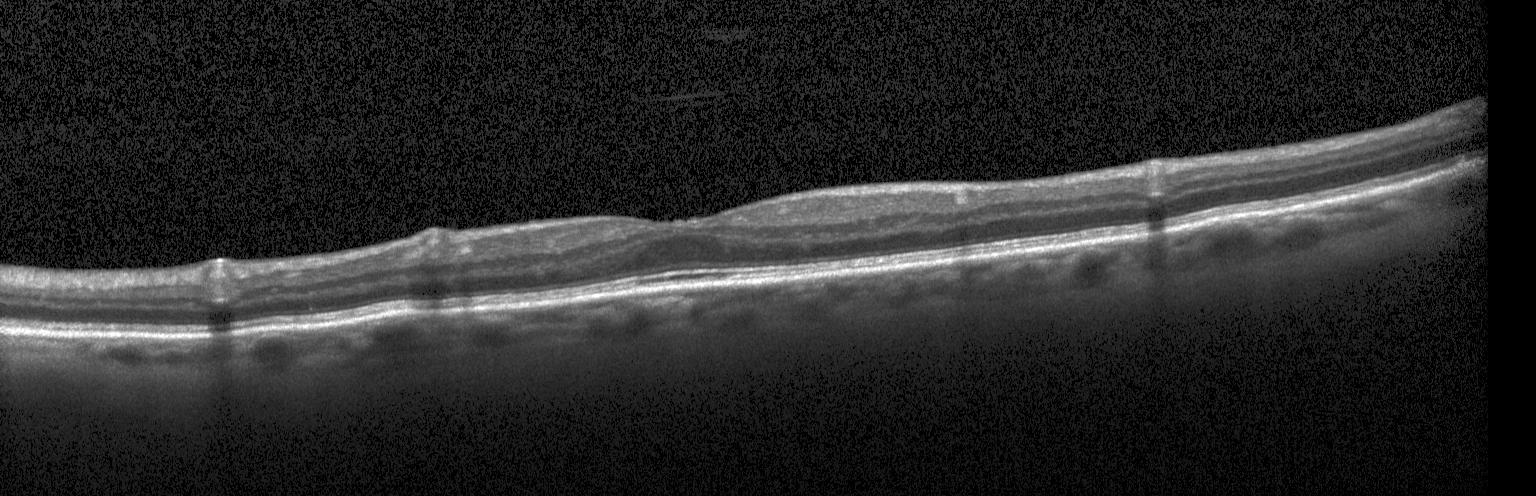
Dx: no choroidal neovascularization, diabetic macular edema, or drusen.